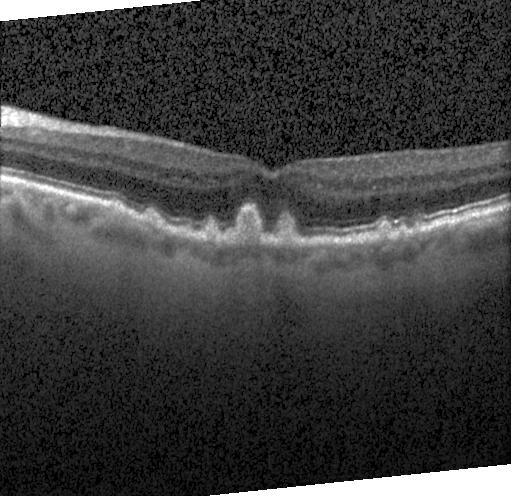
Optical coherence tomography scan. This B-scan demonstrates sub-RPE drusenoid deposits.